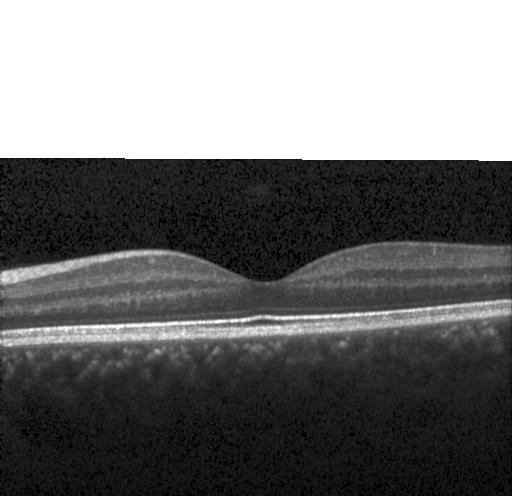 OCT B-scan. Impression: no CNV, no DME, and no drusen.